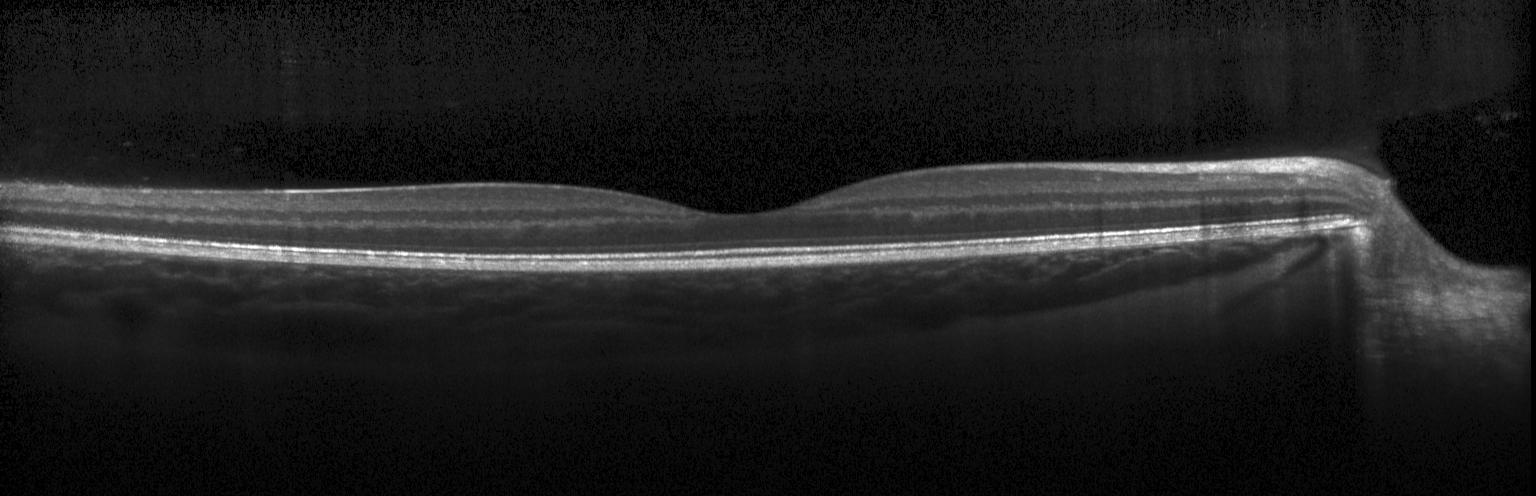 Diagnosis: no evidence of choroidal neovascularization, diabetic macular edema, or drusen.